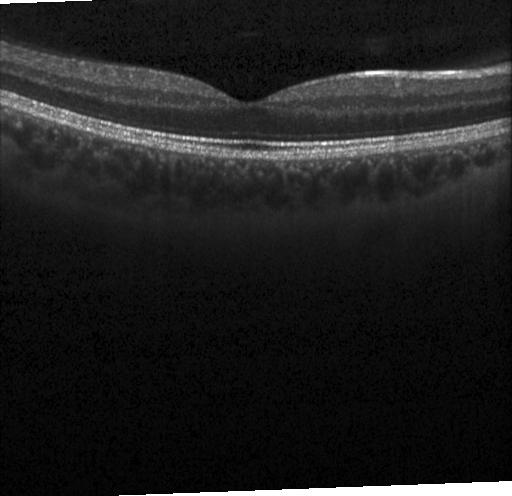 Fovea-centered · optical coherence tomography B-scan.
Diagnosis: neither choroidal neovascularization, diabetic macular edema, nor drusen.